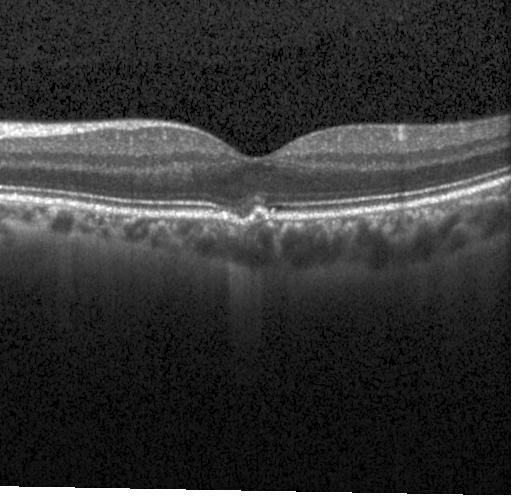
This B-scan demonstrates drusen.